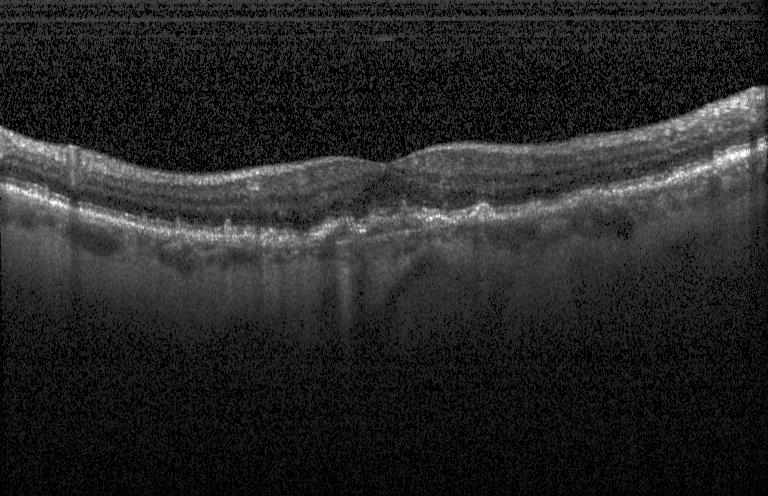

Heidelberg Spectralis OCT system. Retinal OCT cross-section
This B-scan demonstrates a choroidal neovascular membrane.